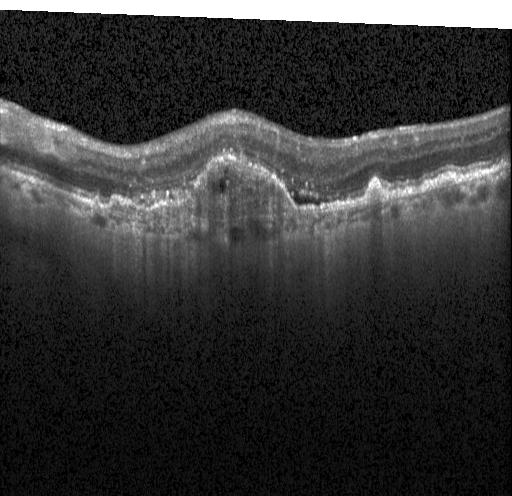
Dx: choroidal neovascularization (CNV).